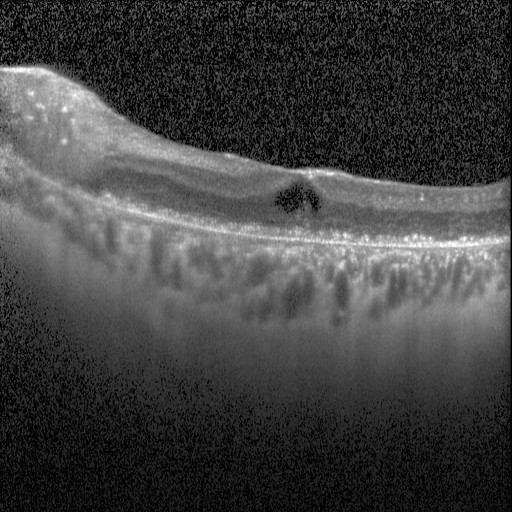 Fovea-centered, retinal OCT B-scan.
The scan shows DME.